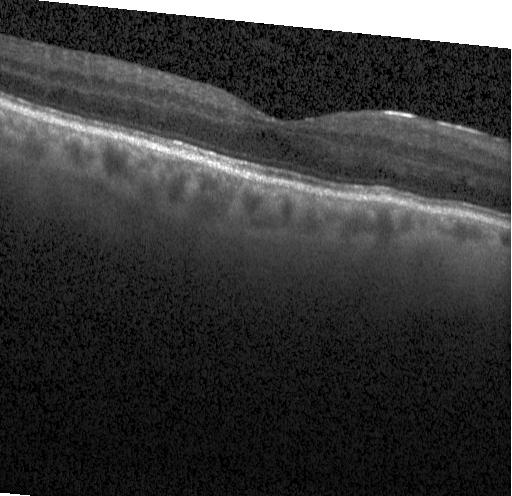

Heidelberg Spectralis, spectral-domain OCT, fovea-centered, optical coherence tomography B-scan.
Macular OCT: no choroidal neovascularization, no diabetic macular edema, and no drusen.